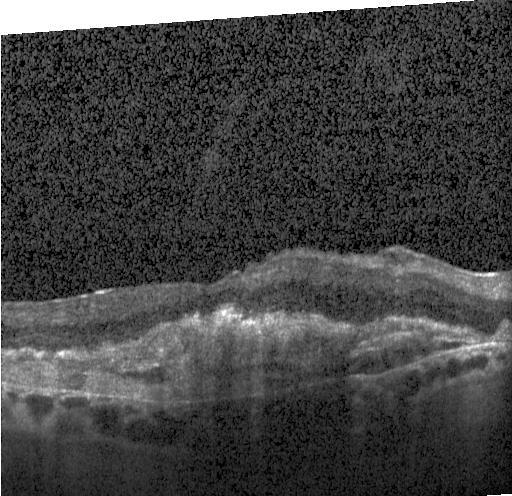 OCT finding: choroidal neovascularization (CNV).